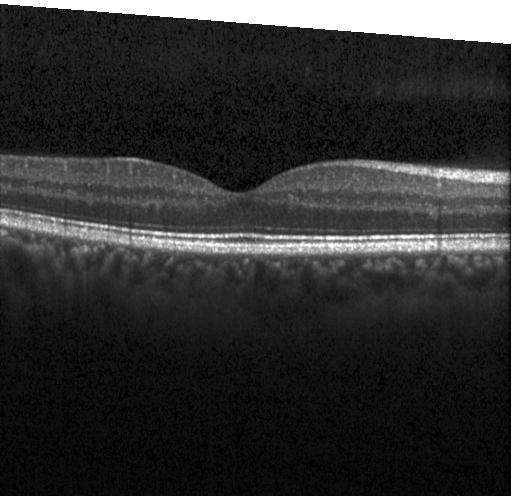 Impression: neither choroidal neovascularization, diabetic macular edema, nor drusen.